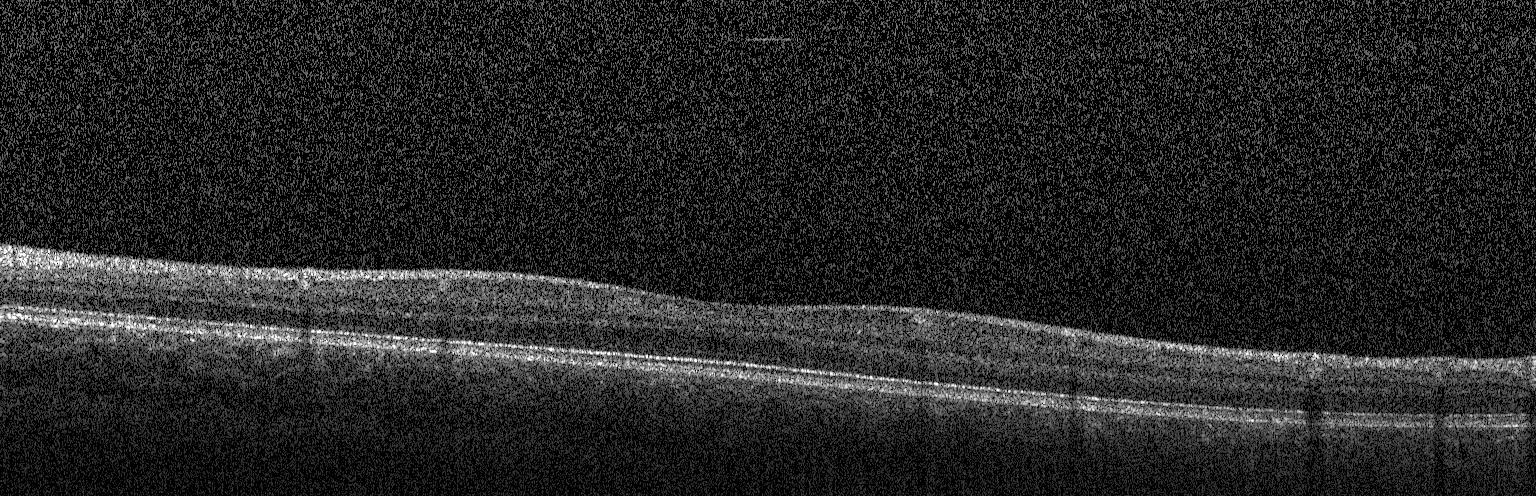 OCT finding: no evidence of choroidal neovascularization, diabetic macular edema, or drusen.